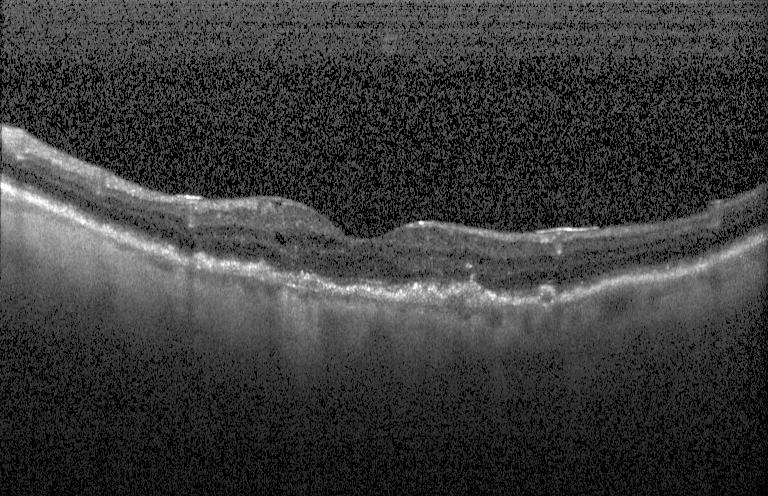
Spectral-domain OCT B-scan: a choroidal neovascular membrane.